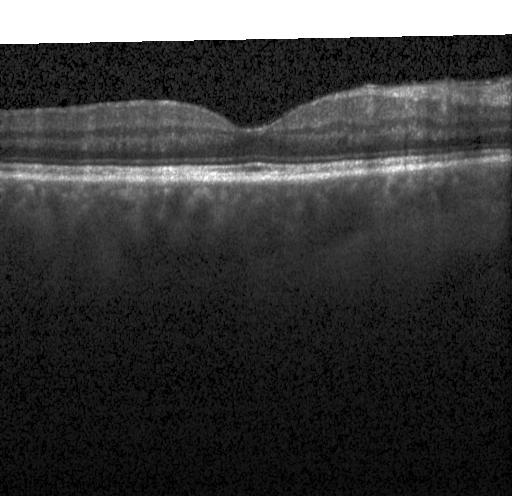
Retinal OCT B-scan. Horizontal scan through the fovea. Instrument: Heidelberg Spectralis — No choroidal neovascularization, no diabetic macular edema, and no drusen.